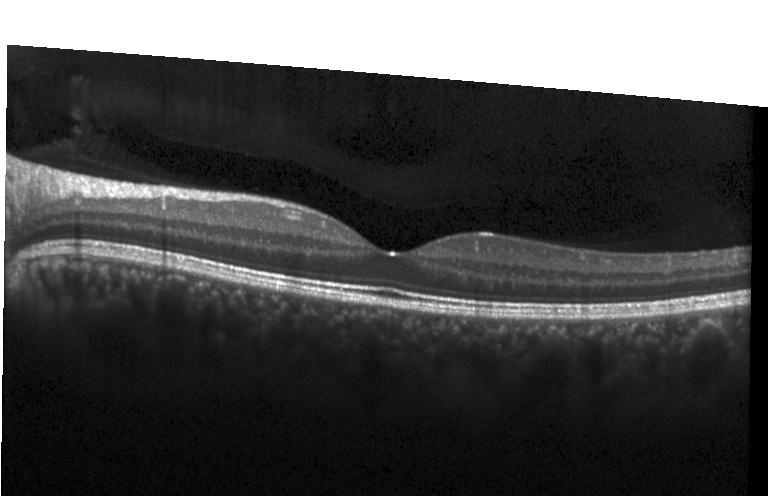

Finding: no choroidal neovascularization, no diabetic macular edema, and no drusen.